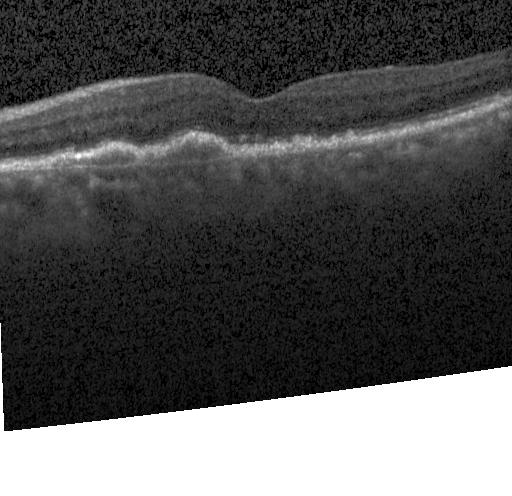 Retinal OCT B-scan
Diagnosis: a choroidal neovascular membrane.